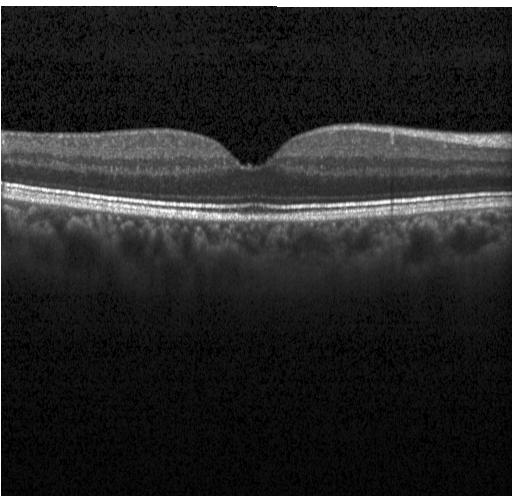
Macular OCT: no choroidal neovascularization, diabetic macular edema, or drusen.